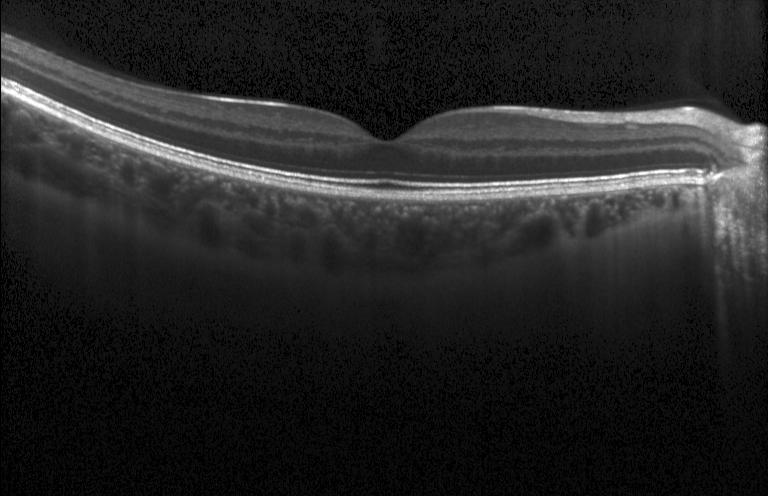
Macular OCT demonstrating no choroidal neovascularization, no diabetic macular edema, and no drusen.